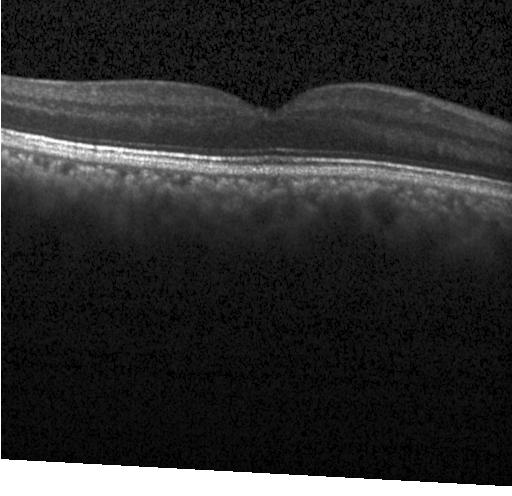 SD-OCT, optical coherence tomography B-scan — Dx: no choroidal neovascularization, no diabetic macular edema, and no drusen.